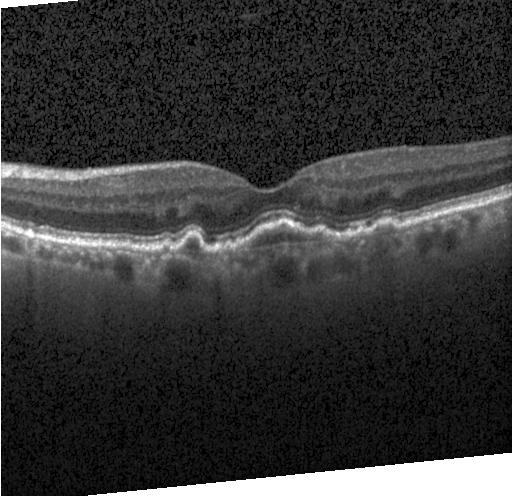 Acquired on a Heidelberg Spectralis, optical coherence tomography B-scan. Choroidal neovascularization.